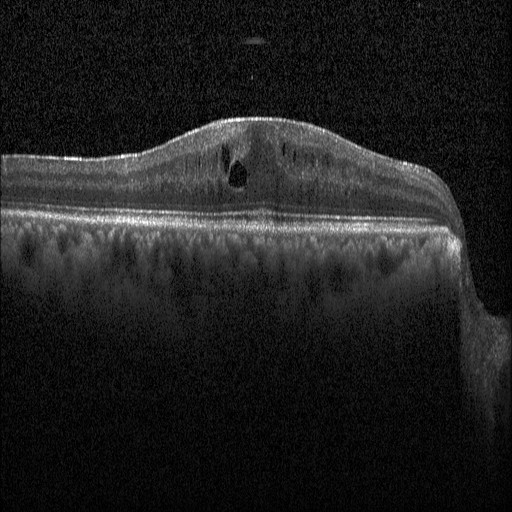 Macular OCT demonstrating diabetic macular edema.